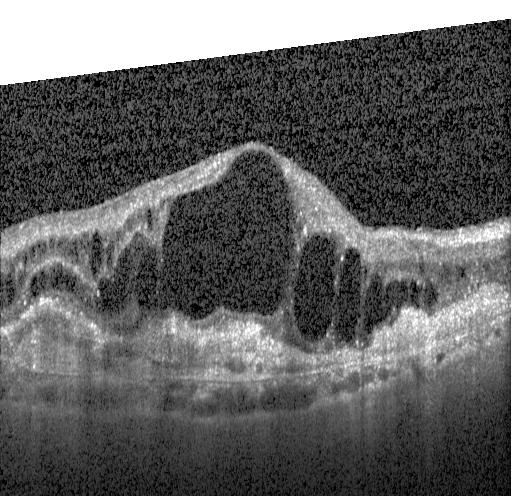 Spectral-domain OCT · optical coherence tomography scan · through the macula. Impression: a choroidal neovascular membrane.